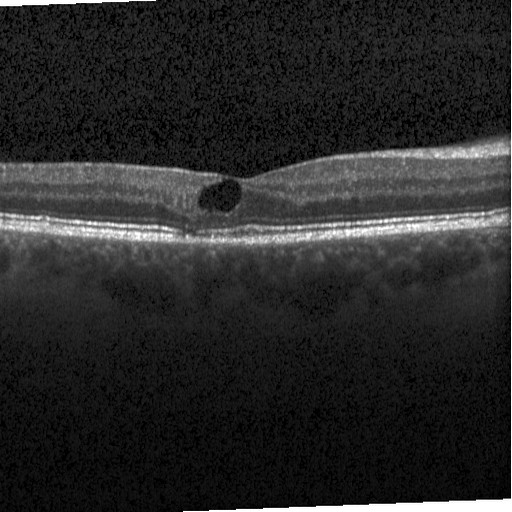

Spectral-domain OCT, optical coherence tomography scan, Heidelberg Spectralis, through the macula. Dx: DME.